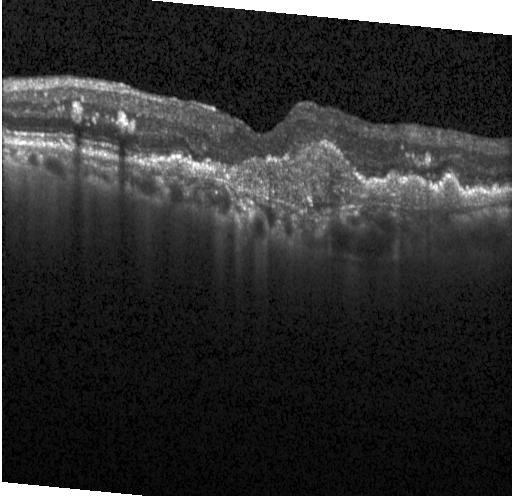
Retinal OCT B-scan; spectral-domain OCT
Finding: CNV.